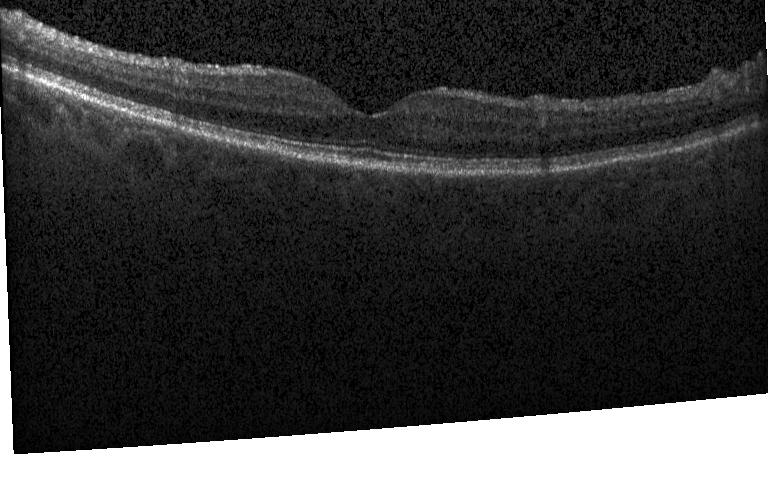

Optical coherence tomography B-scan.
Finding: neither choroidal neovascularization, diabetic macular edema, nor drusen.